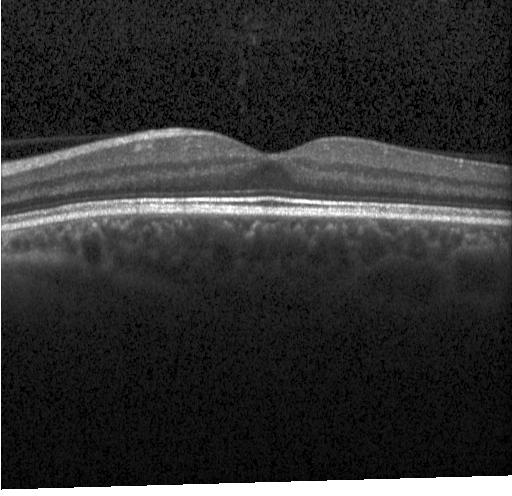

Optical coherence tomography B-scan
Finding: no choroidal neovascularization, no diabetic macular edema, and no drusen.